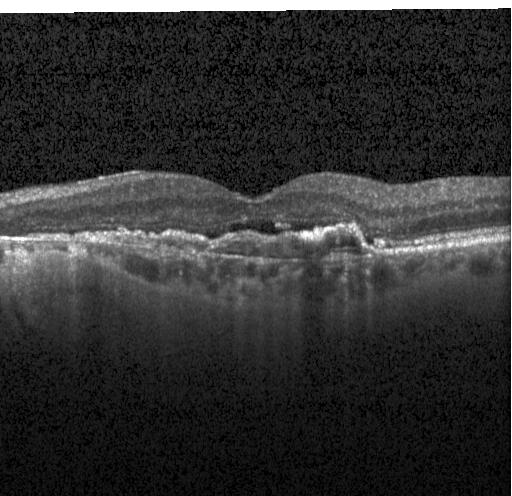

This B-scan demonstrates CNV.